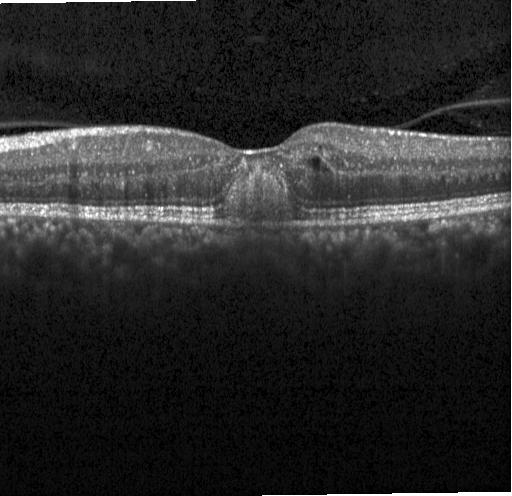 OCT finding: a choroidal neovascular membrane.